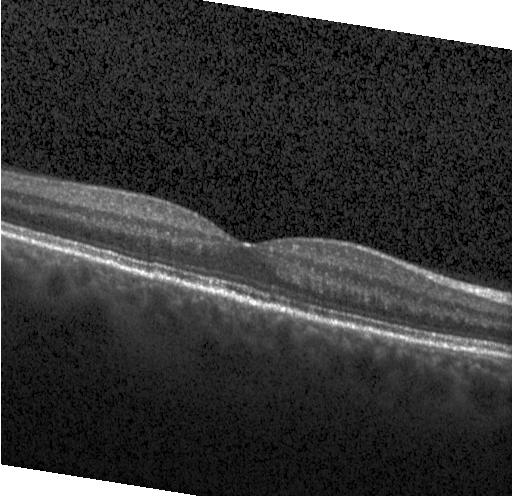 Retinal OCT B-scan.
The scan shows no CNV, DME, or drusen.